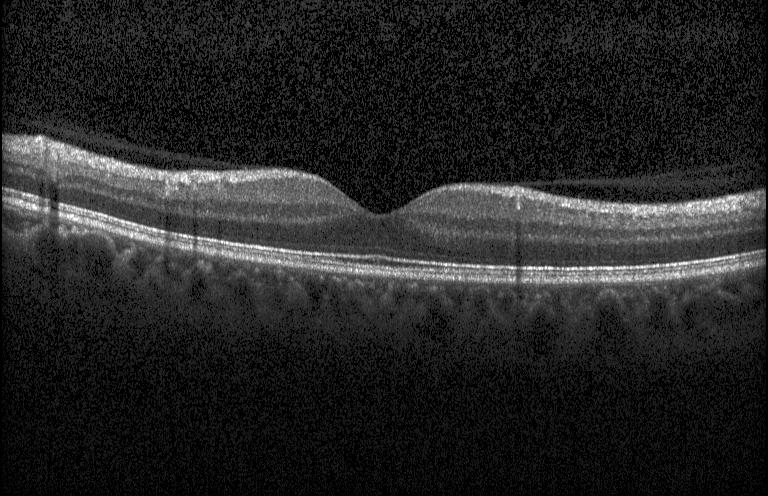
Acquired on a Heidelberg Spectralis, retinal OCT cross-section, spectral-domain optical coherence tomography
This B-scan demonstrates no evidence of choroidal neovascularization, diabetic macular edema, or drusen.